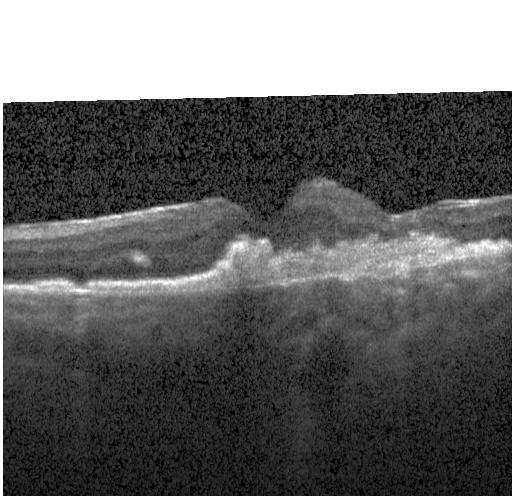

Heidelberg Spectralis, OCT line scan
Impression: CNV.